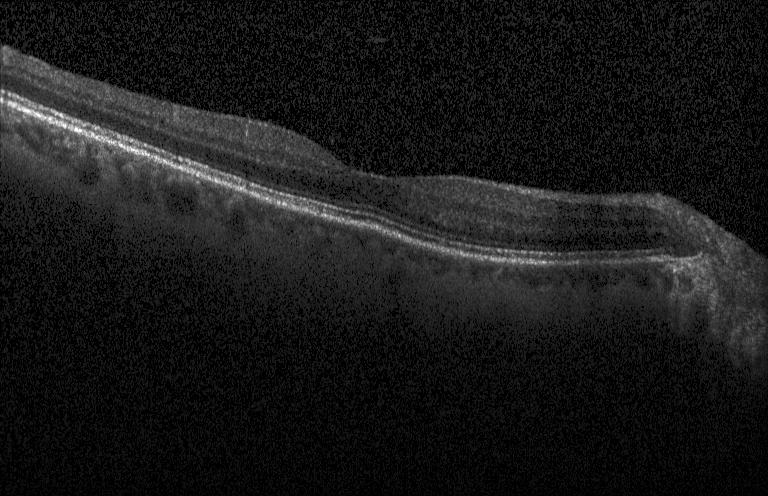
Finding: no CNV, DME, or drusen.